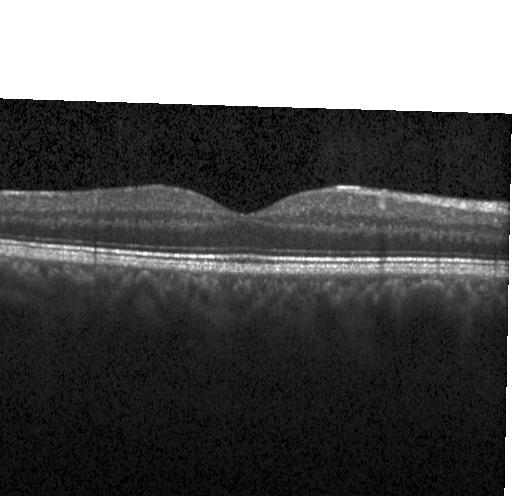 Assessment: no choroidal neovascularization, no diabetic macular edema, and no drusen.